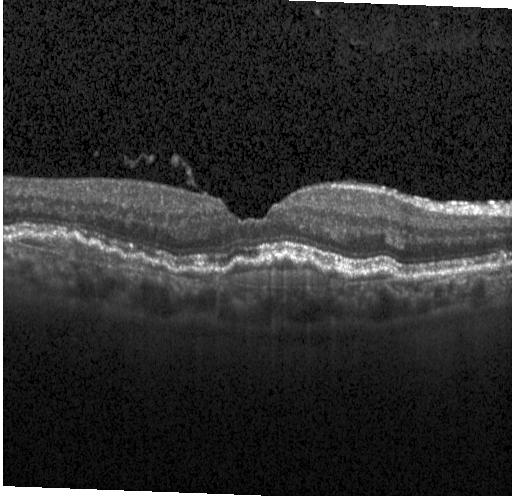

Spectral-domain optical coherence tomography. Retinal OCT cross-section. Centered on the fovea.
A choroidal neovascular membrane.